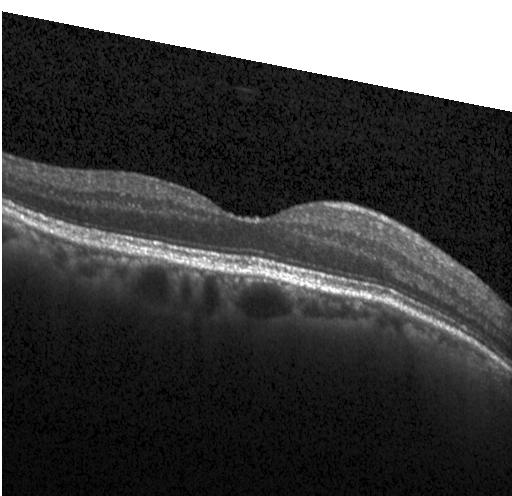 Acquired on a Heidelberg Spectralis; OCT B-scan.
Dx: no CNV, no DME, and no drusen.